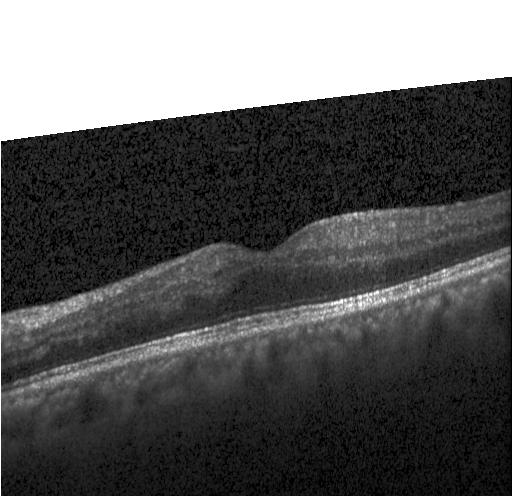 Finding: no CNV, DME, or drusen.